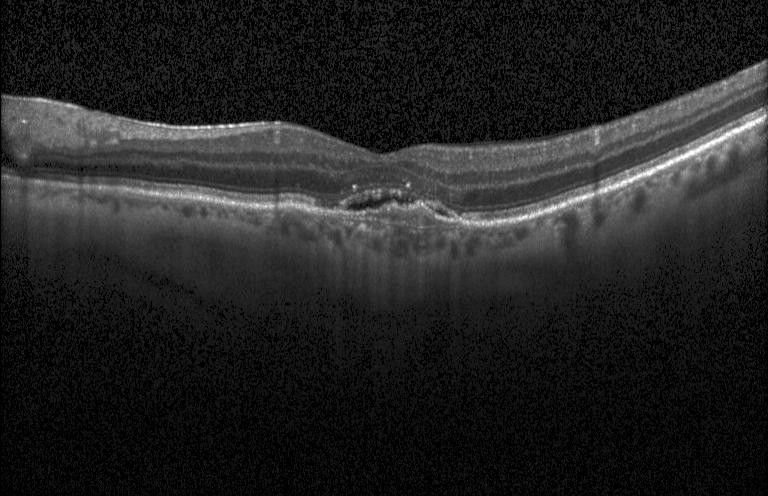 OCT line scan, acquired on a Heidelberg Spectralis, spectral-domain OCT, horizontal scan through the fovea — A choroidal neovascular membrane.